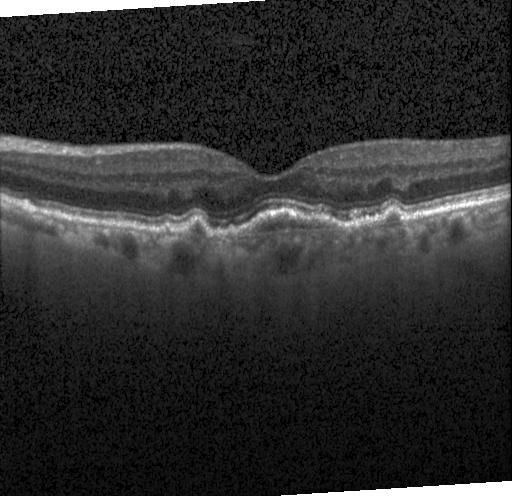
Optical coherence tomography B-scan
Finding: CNV.